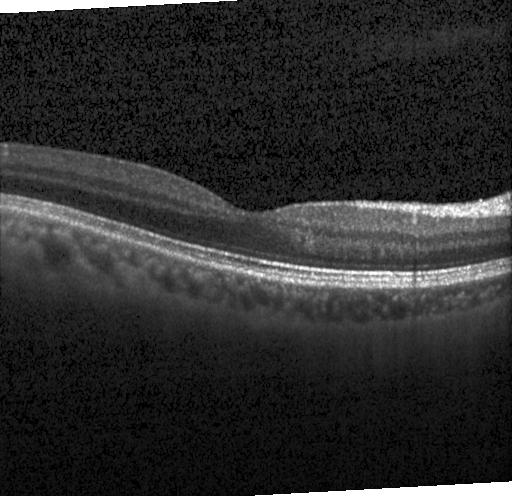 Spectral-domain optical coherence tomography; through the macula; OCT line scan.
Impression: no CNV, DME, or drusen.